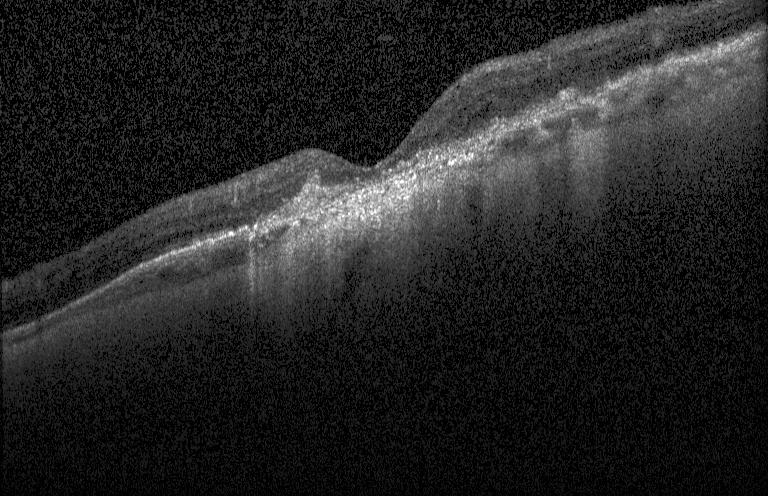

SD-OCT, macular scan, retinal OCT B-scan
Choroidal neovascularization.